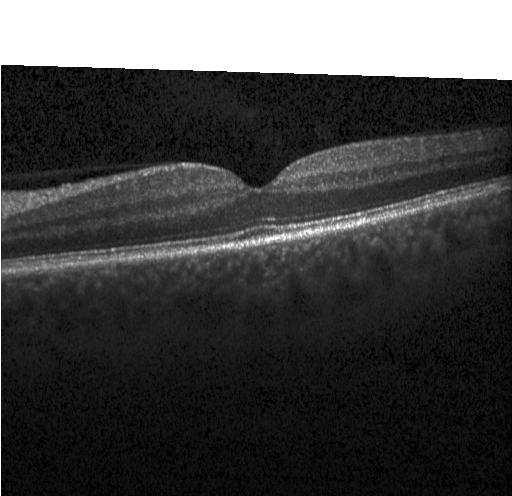
OCT B-scan
Impression: neither choroidal neovascularization, diabetic macular edema, nor drusen.